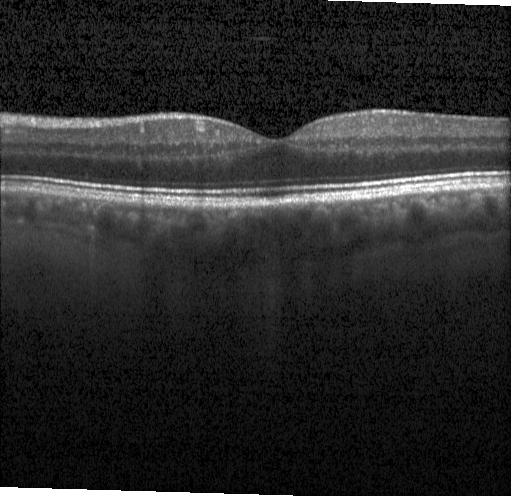 Retinal OCT cross-section · Heidelberg Spectralis.
The scan shows no choroidal neovascularization, no diabetic macular edema, and no drusen.